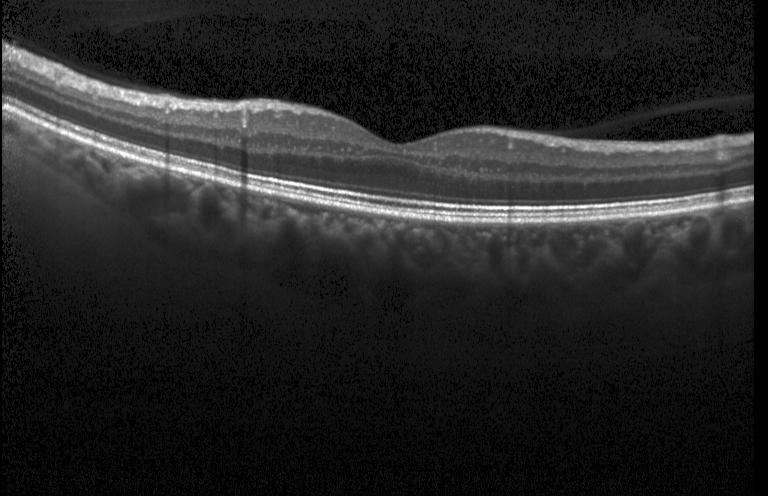
Through the macula; SD-OCT; retinal OCT cross-section.
Impression: no CNV, no DME, and no drusen.